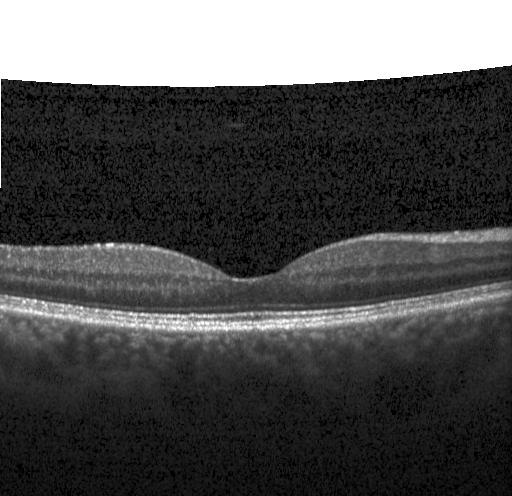

OCT B-scan showing no choroidal neovascularization, diabetic macular edema, or drusen.